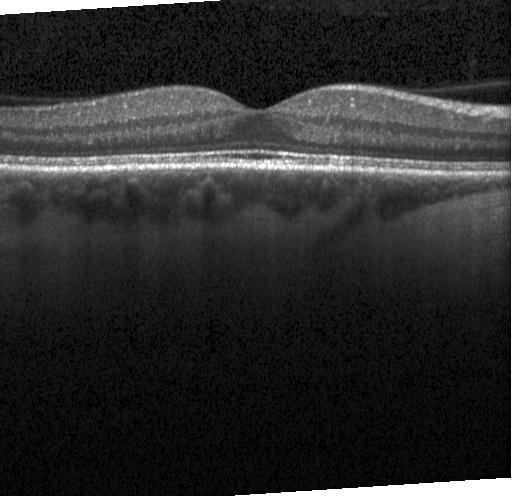 Diagnosis: no CNV, DME, or drusen.